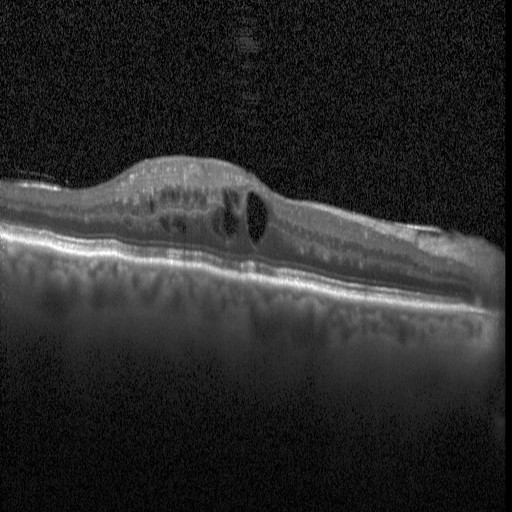 Optical coherence tomography B-scan · Heidelberg Spectralis. Diabetic macular edema.